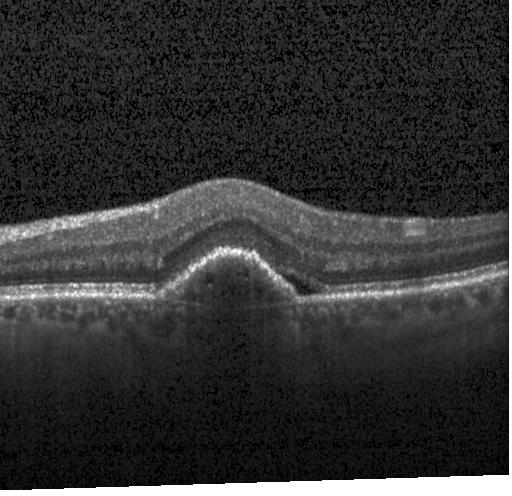

Horizontal scan through the fovea, retinal OCT B-scan.
OCT finding: CNV.